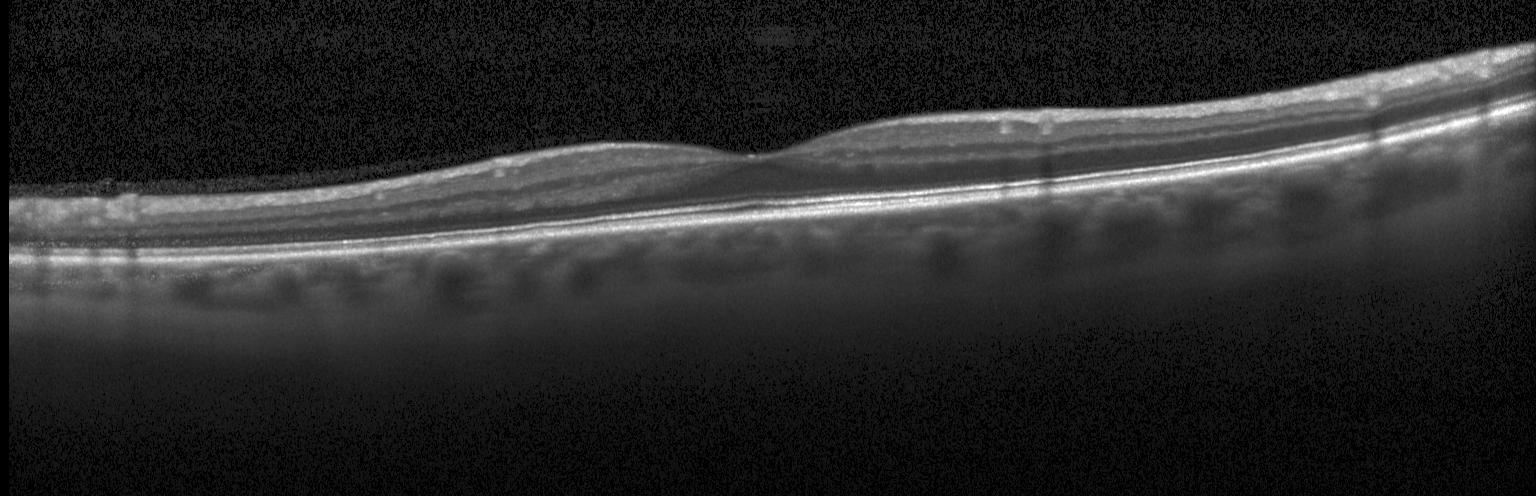
Impression: neither CNV, DME, nor drusen.